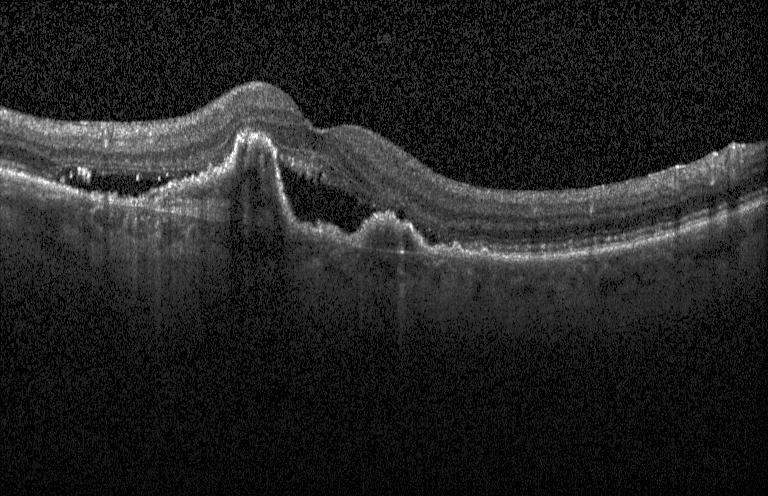 Assessment: choroidal neovascularization.